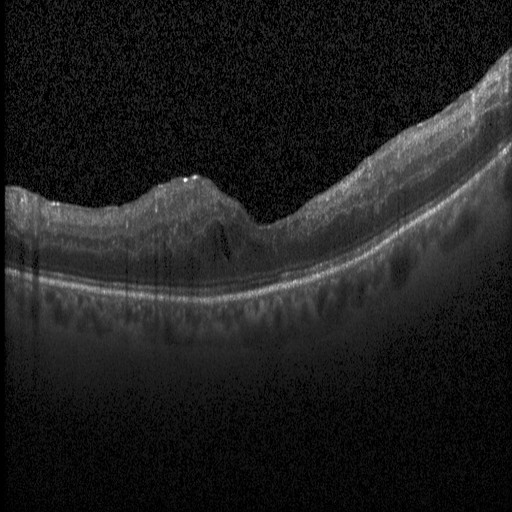
OCT line scan
Finding: DME.